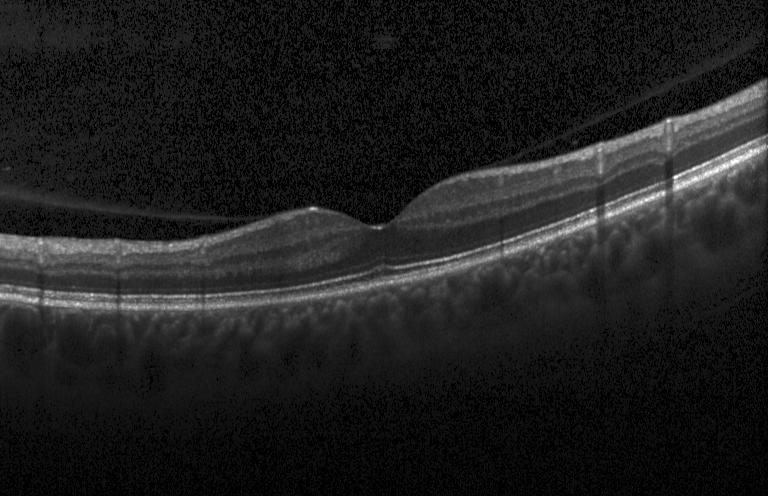

Retinal OCT B-scan. Diagnosis: no choroidal neovascularization, no diabetic macular edema, and no drusen.